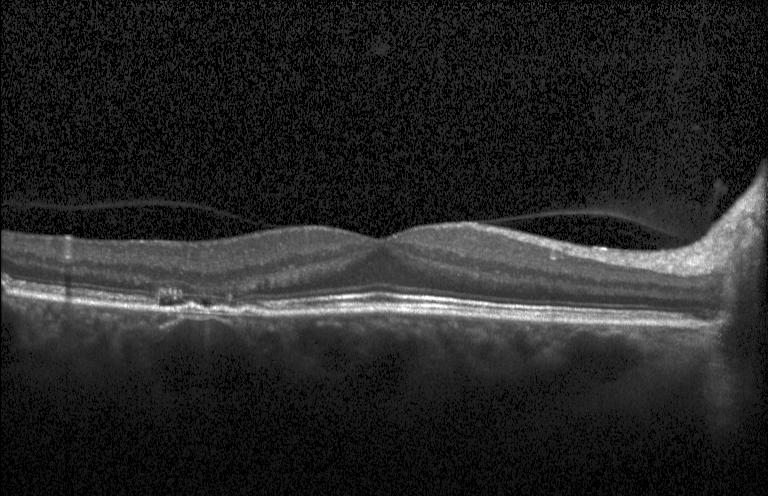 Horizontal scan through the fovea, SD-OCT, retinal OCT B-scan. Impression: CNV.